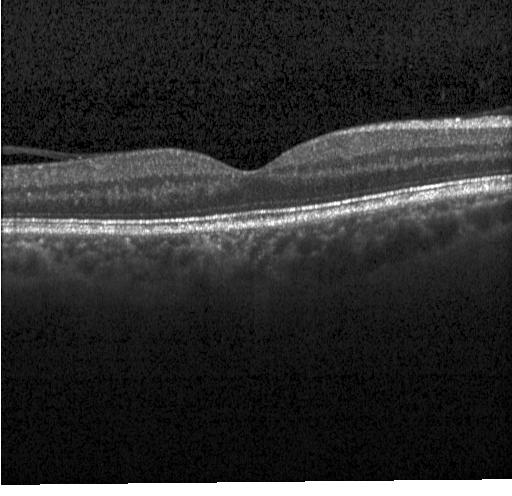

Heidelberg Spectralis OCT system · centered on the fovea · spectral-domain optical coherence tomography · retinal OCT B-scan.
Finding: no choroidal neovascularization, diabetic macular edema, or drusen.